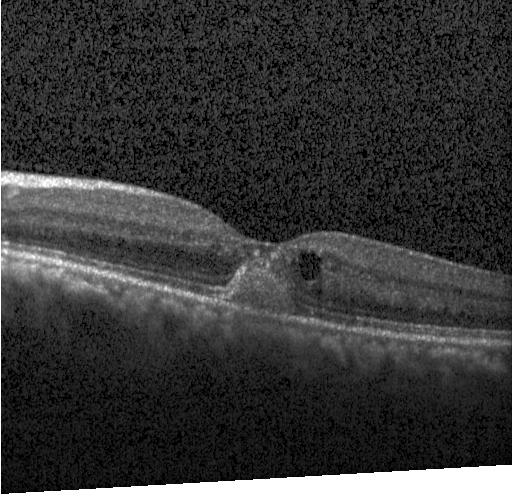
Acquired on a Heidelberg Spectralis. Spectral-domain OCT. Retinal OCT B-scan. Horizontal scan through the fovea. Macular OCT: CNV.